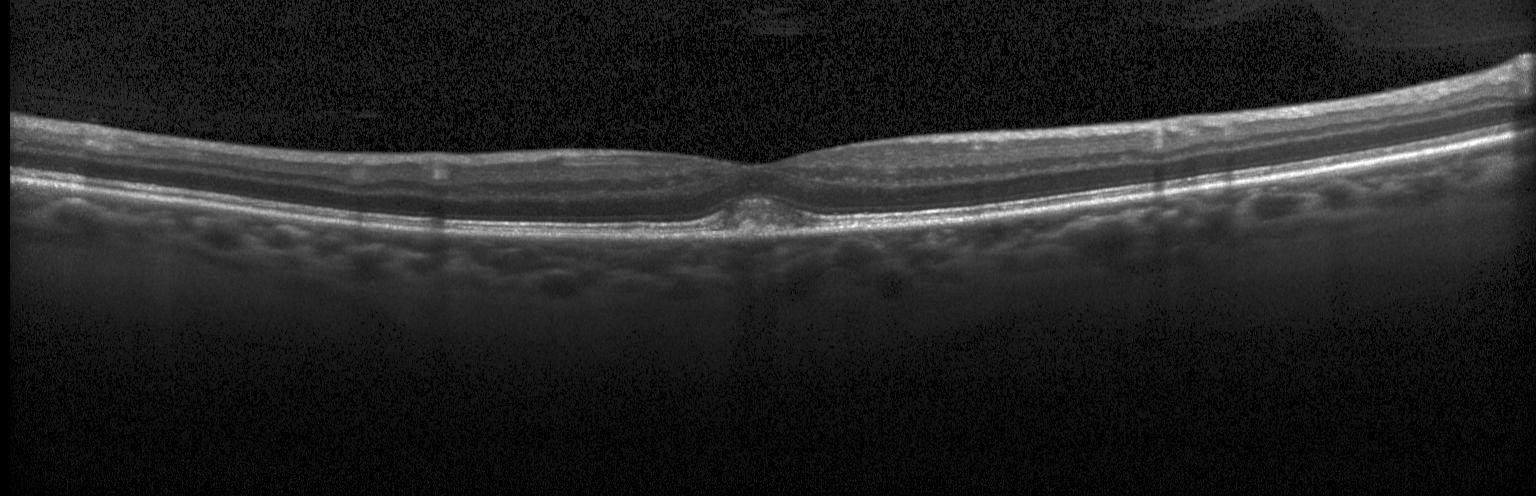

Retinal OCT cross-section showing sub-RPE drusenoid deposits.